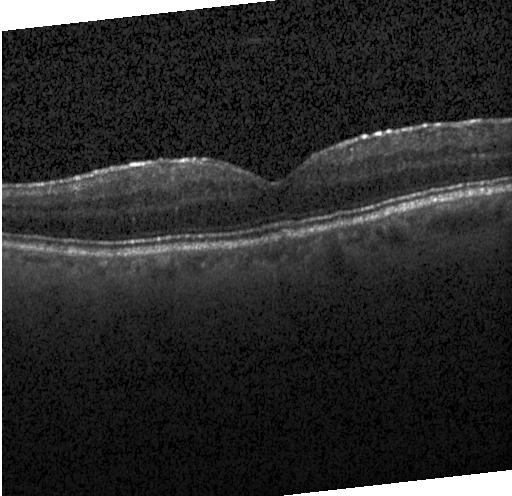 Diagnosis: no evidence of choroidal neovascularization, diabetic macular edema, or drusen.